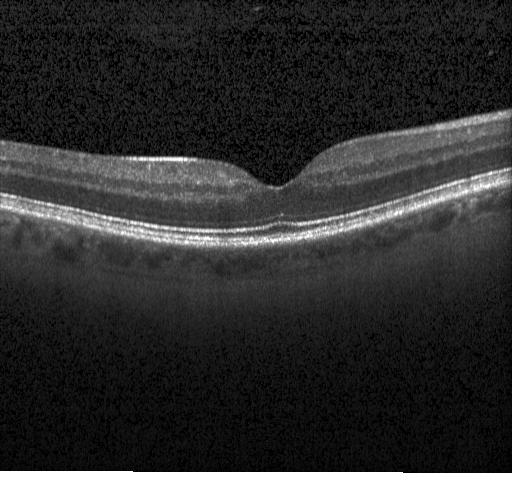

Heidelberg Spectralis, optical coherence tomography B-scan, spectral-domain OCT
Dx: no choroidal neovascularization, diabetic macular edema, or drusen.